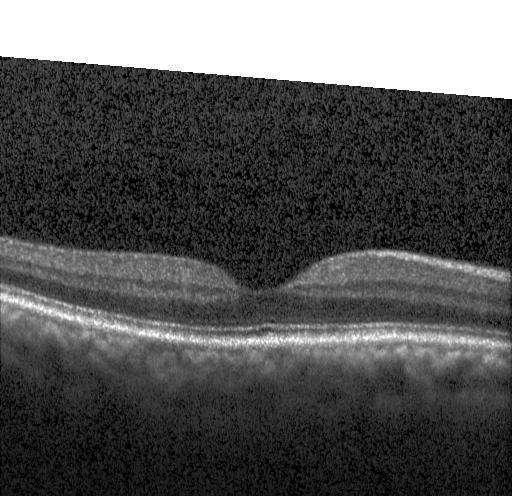
OCT scan showing neither CNV, DME, nor drusen.